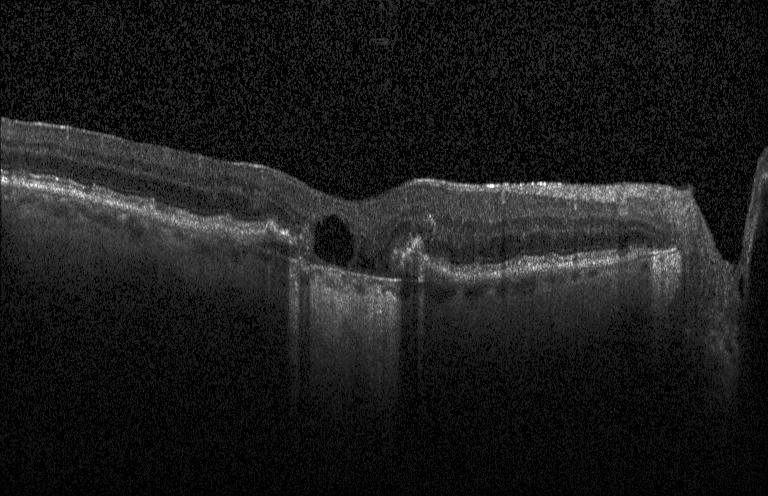 Macular OCT demonstrating CNV.